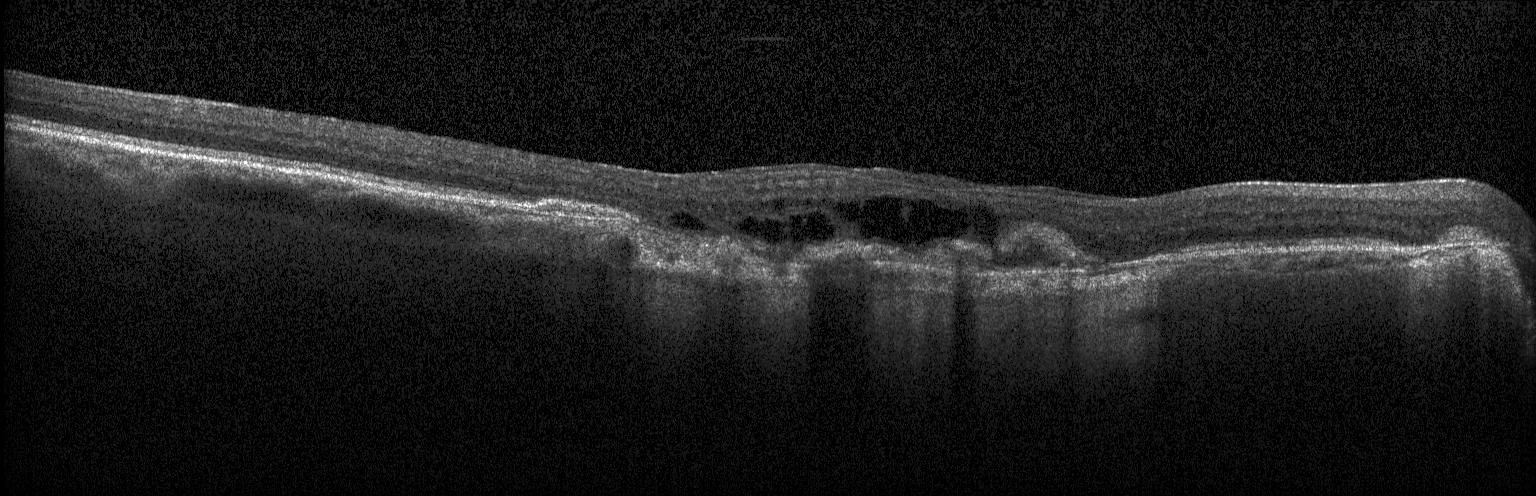 Acquired on a Heidelberg Spectralis · spectral-domain OCT · OCT B-scan. Finding: a choroidal neovascular membrane.